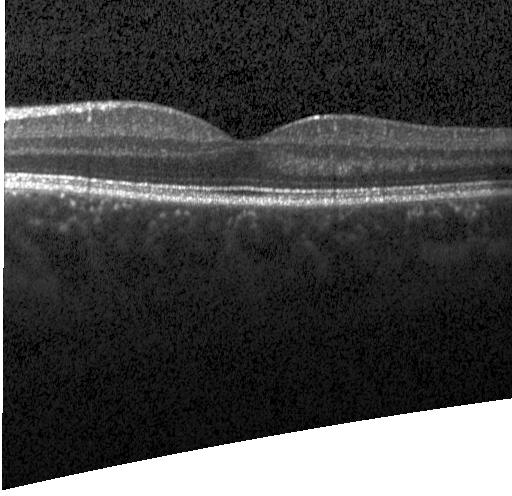
Through the macula, OCT B-scan, acquired on a Heidelberg Spectralis — No evidence of choroidal neovascularization, diabetic macular edema, or drusen.